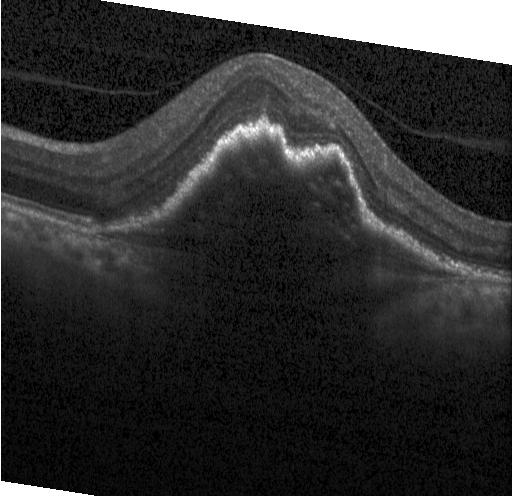
Horizontal scan through the fovea · spectral-domain OCT · retinal OCT B-scan — Diagnosis: a choroidal neovascular membrane.